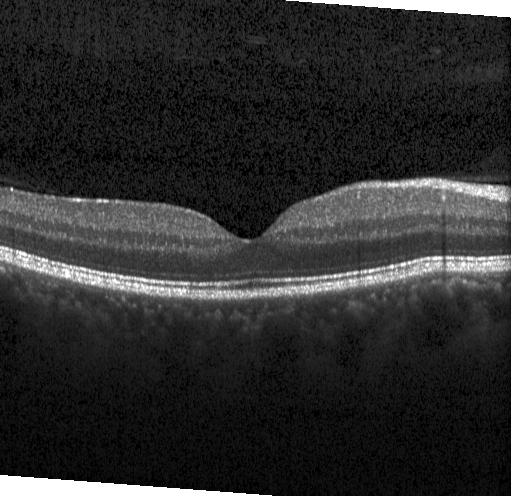 Retinal OCT B-scan; acquired on a Heidelberg Spectralis; through the macula. Macular OCT: no evidence of choroidal neovascularization, diabetic macular edema, or drusen.